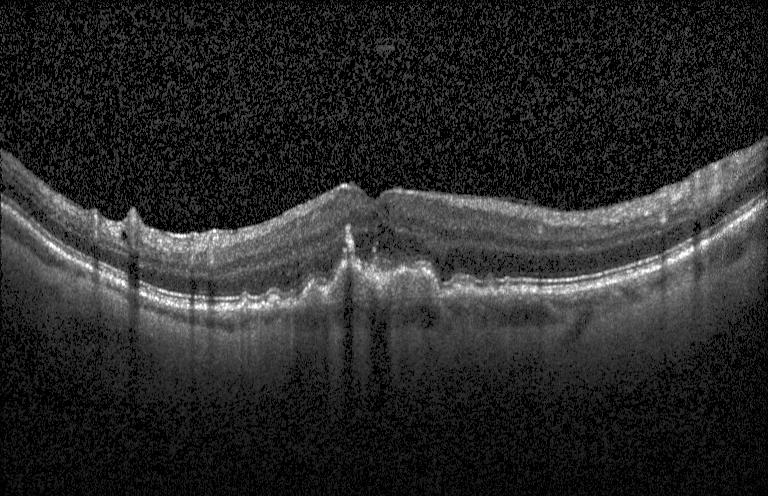

Heidelberg Spectralis, retinal OCT B-scan, spectral-domain OCT, macular scan
Diagnosis: drusen.